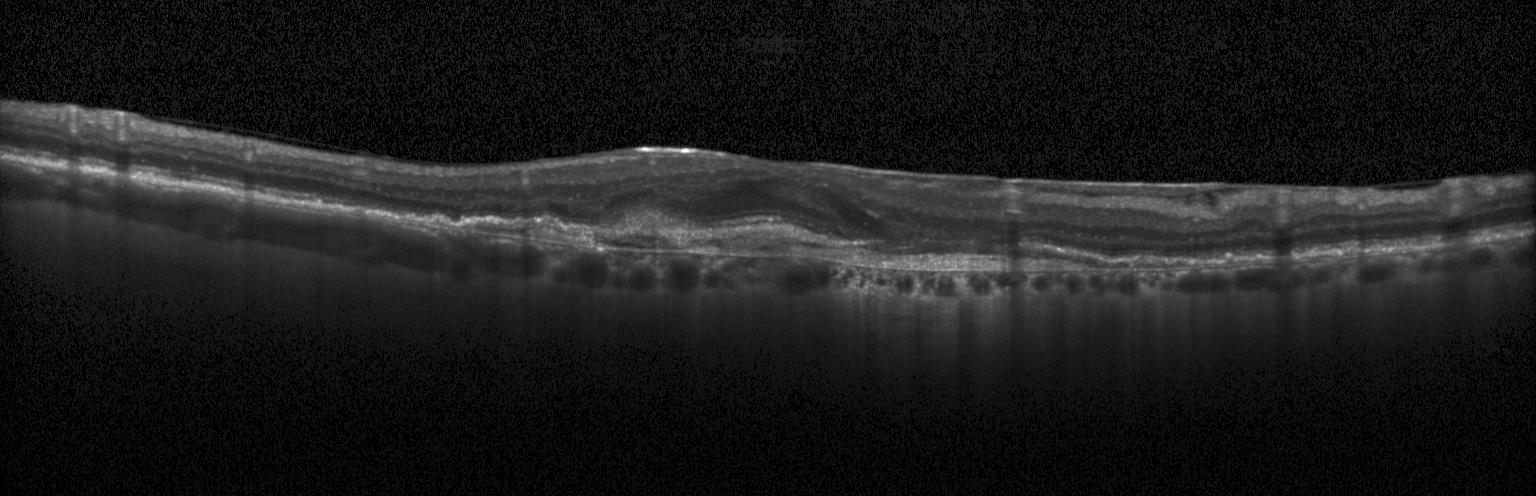
Instrument: Heidelberg Spectralis. Spectral-domain optical coherence tomography. Optical coherence tomography B-scan. Macular scan — Finding: choroidal neovascularization (CNV).